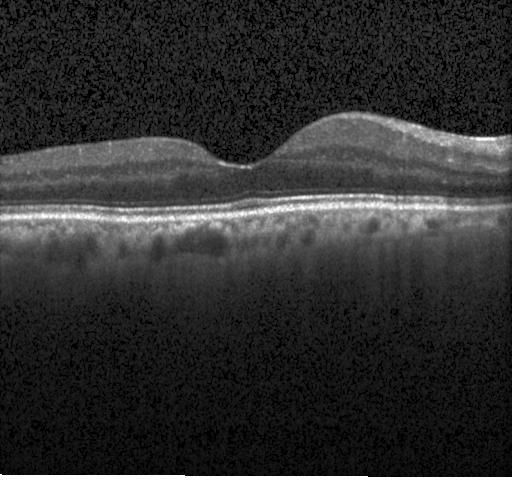

OCT scan showing no CNV, DME, or drusen.